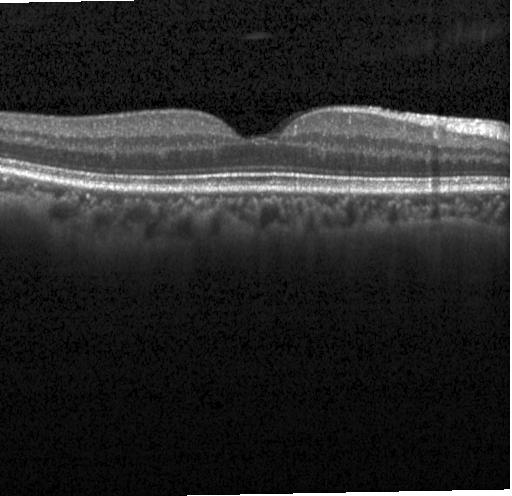 Diagnosis: neither choroidal neovascularization, diabetic macular edema, nor drusen.